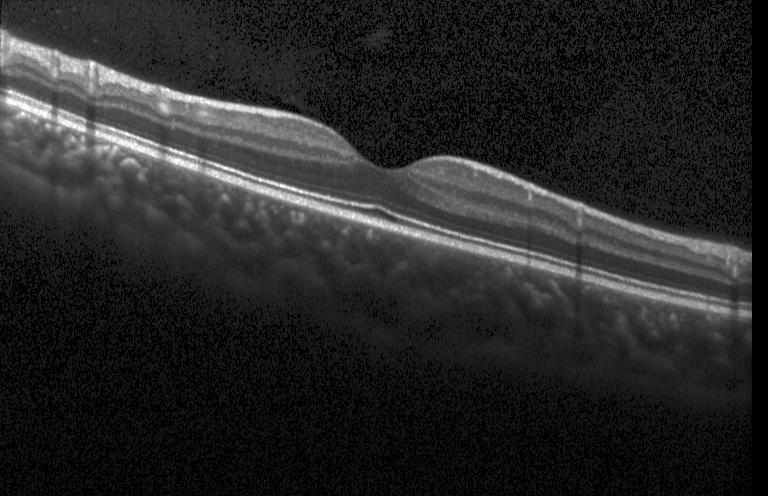

OCT B-scan
Impression: no choroidal neovascularization, no diabetic macular edema, and no drusen.